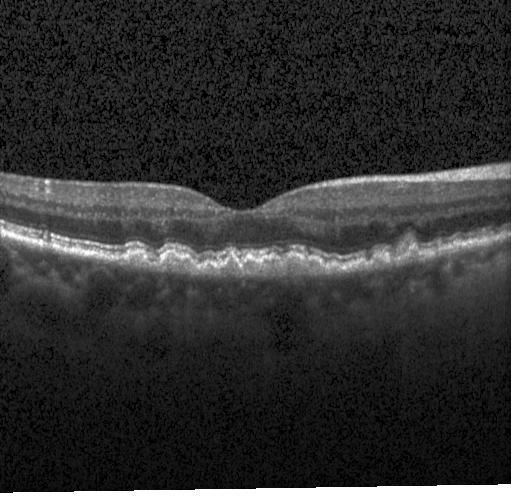

OCT B-scan. The scan shows drusen.